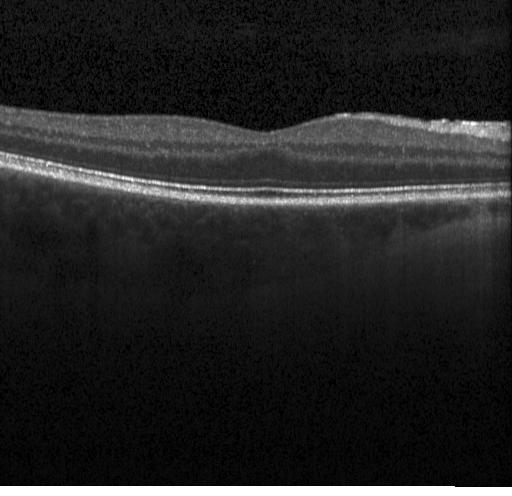

Instrument: Heidelberg Spectralis. Fovea-centered. Optical coherence tomography scan. Spectral-domain OCT
This B-scan demonstrates no choroidal neovascularization, diabetic macular edema, or drusen.